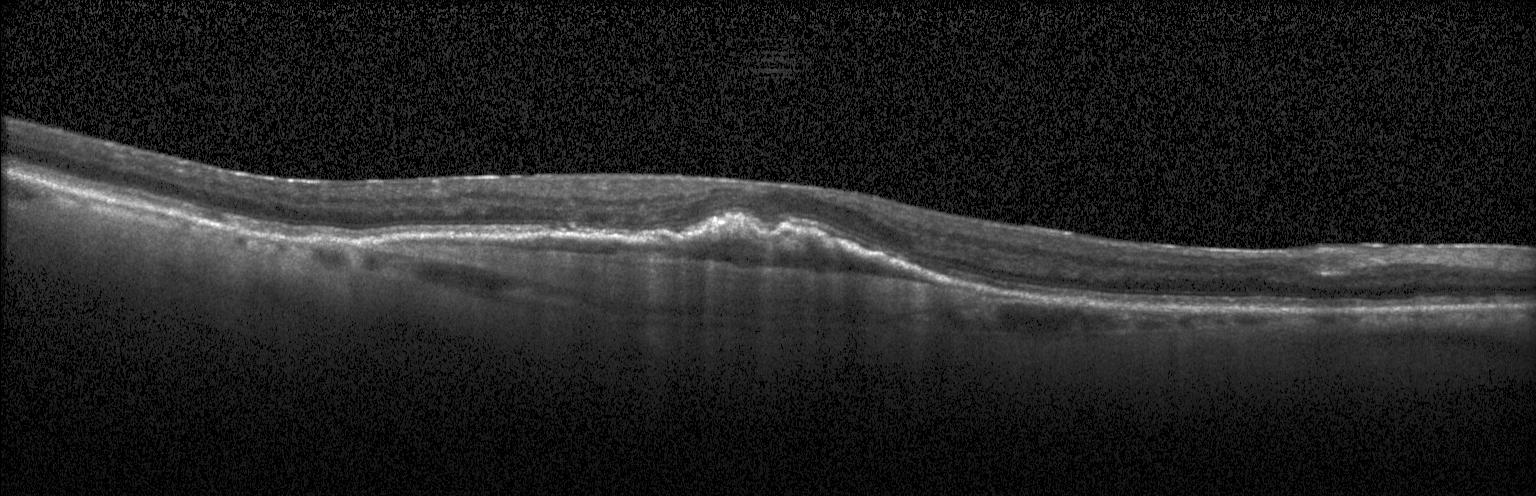

Retinal OCT B-scan.
This B-scan demonstrates CNV.